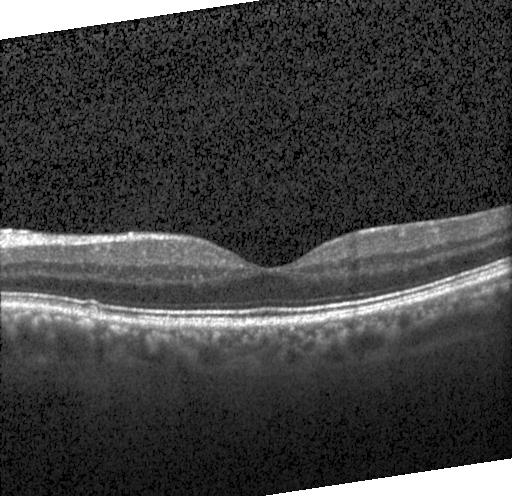

Dx: sub-RPE drusenoid deposits.